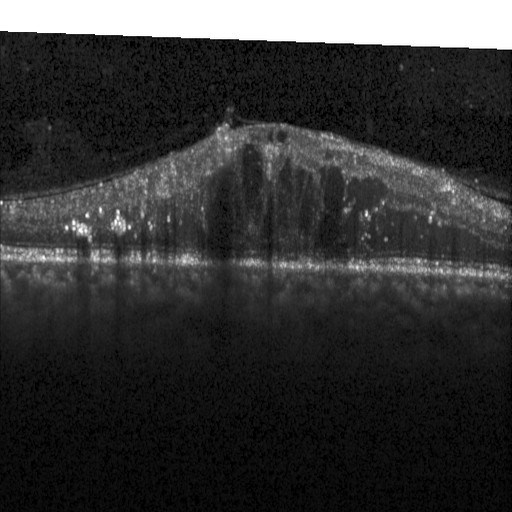 OCT B-scan showing diabetic macular edema.